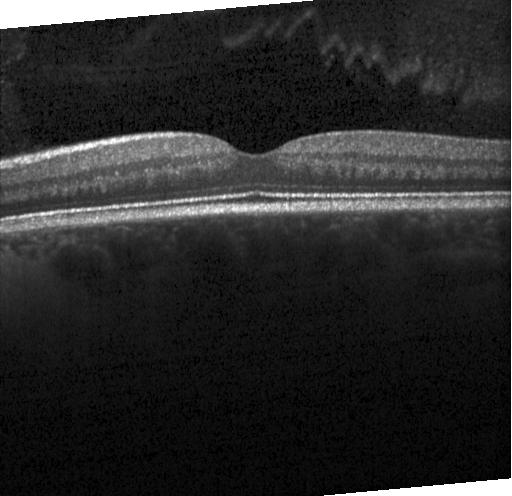
OCT B-scan showing no choroidal neovascularization, no diabetic macular edema, and no drusen.